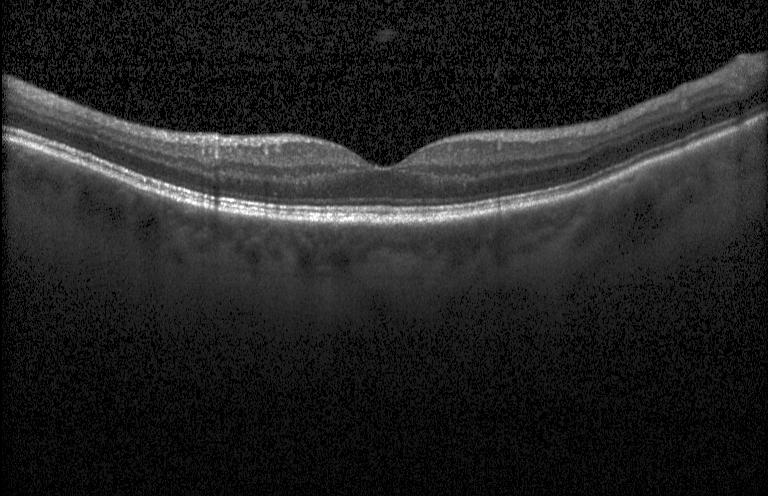 Finding: no evidence of choroidal neovascularization, diabetic macular edema, or drusen.